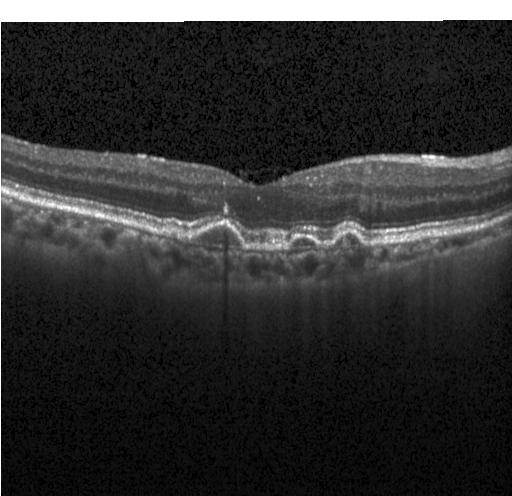 The scan shows a choroidal neovascular membrane.